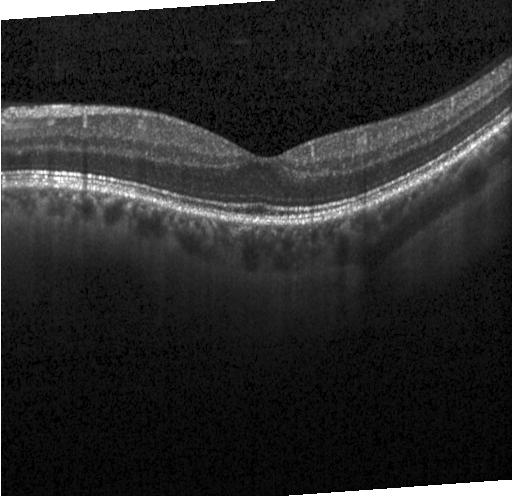
Retinal OCT cross-section, fovea-centered, acquired on a Heidelberg Spectralis.
Impression: neither CNV, DME, nor drusen.